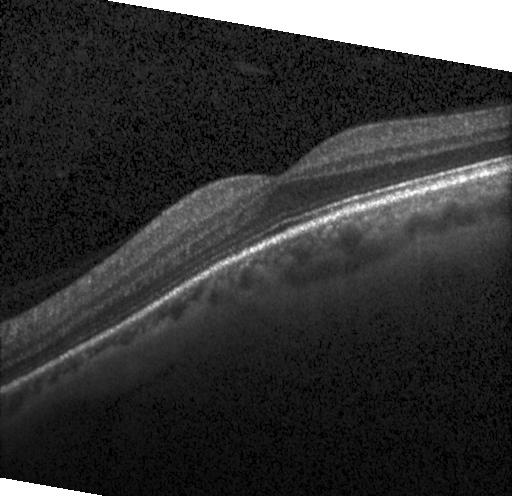 Retinal OCT B-scan, macular scan
Macular OCT: no CNV, DME, or drusen.